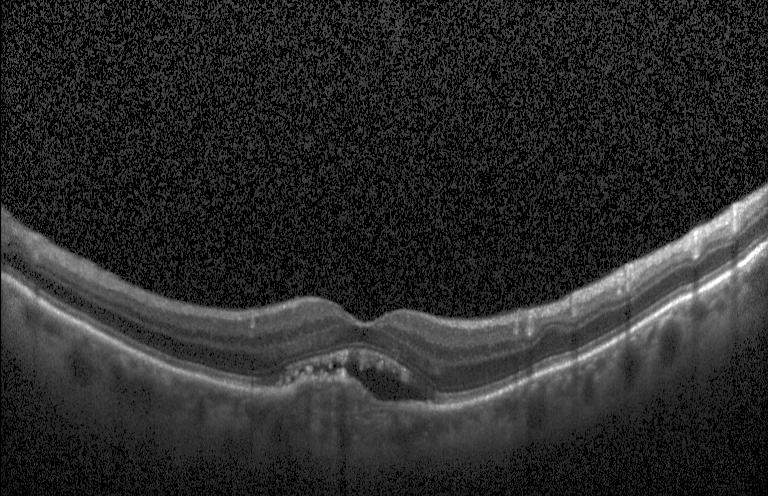

Dx: choroidal neovascularization.